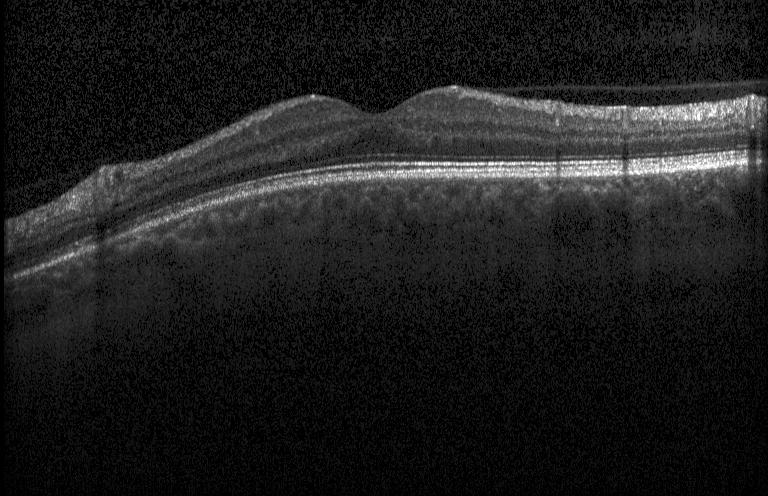
Centered on the fovea; retinal OCT cross-section; Heidelberg Spectralis OCT system
The scan shows neither choroidal neovascularization, diabetic macular edema, nor drusen.